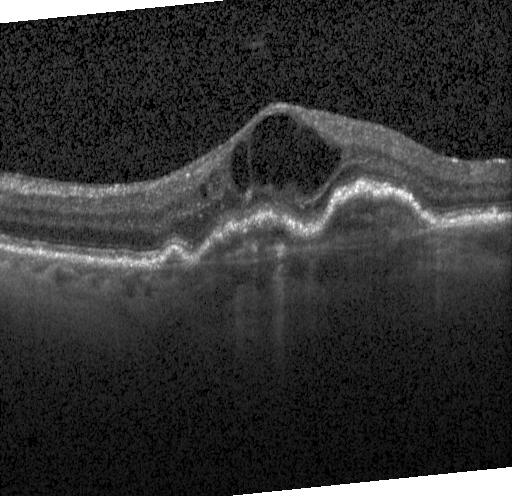

Heidelberg Spectralis · optical coherence tomography B-scan
Diagnosis: a choroidal neovascular membrane.